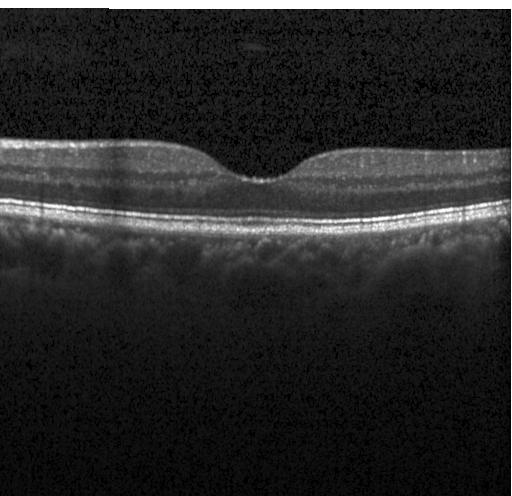

Through the macula, optical coherence tomography scan. The scan shows no CNV, DME, or drusen.